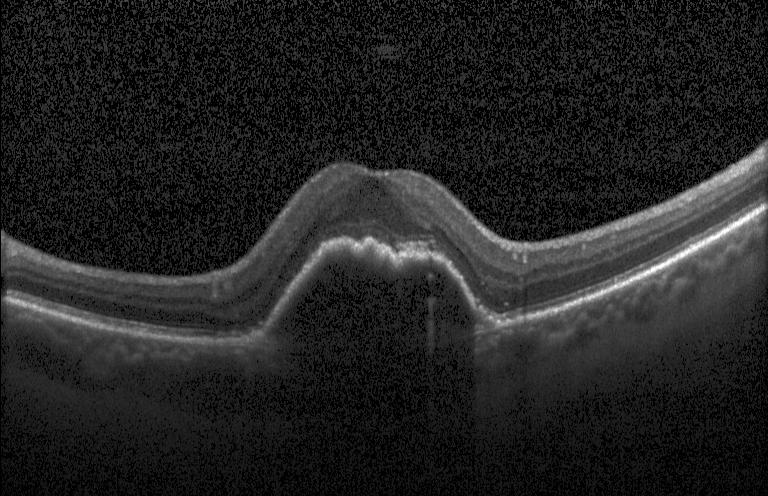
Horizontal scan through the fovea, spectral-domain OCT, instrument: Heidelberg Spectralis, optical coherence tomography scan.
Macular OCT: a choroidal neovascular membrane.